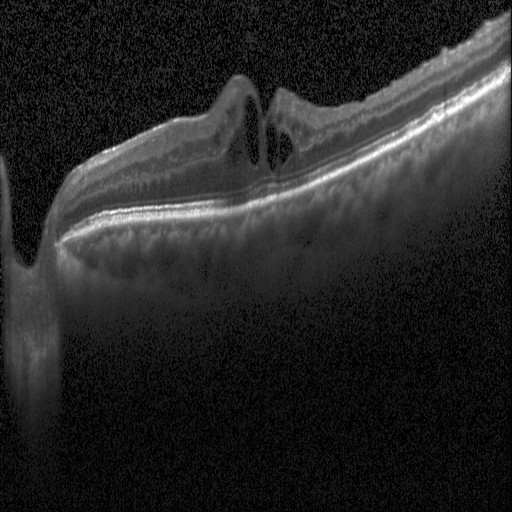
Optical coherence tomography scan — Macular OCT: diabetic macular edema (DME).